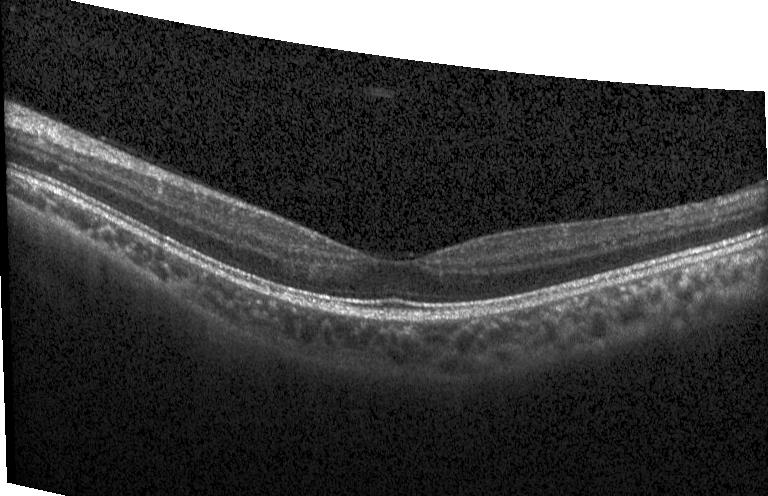

Horizontal scan through the fovea · retinal OCT cross-section · acquired on a Heidelberg Spectralis. Dx: no evidence of CNV, DME, or drusen.